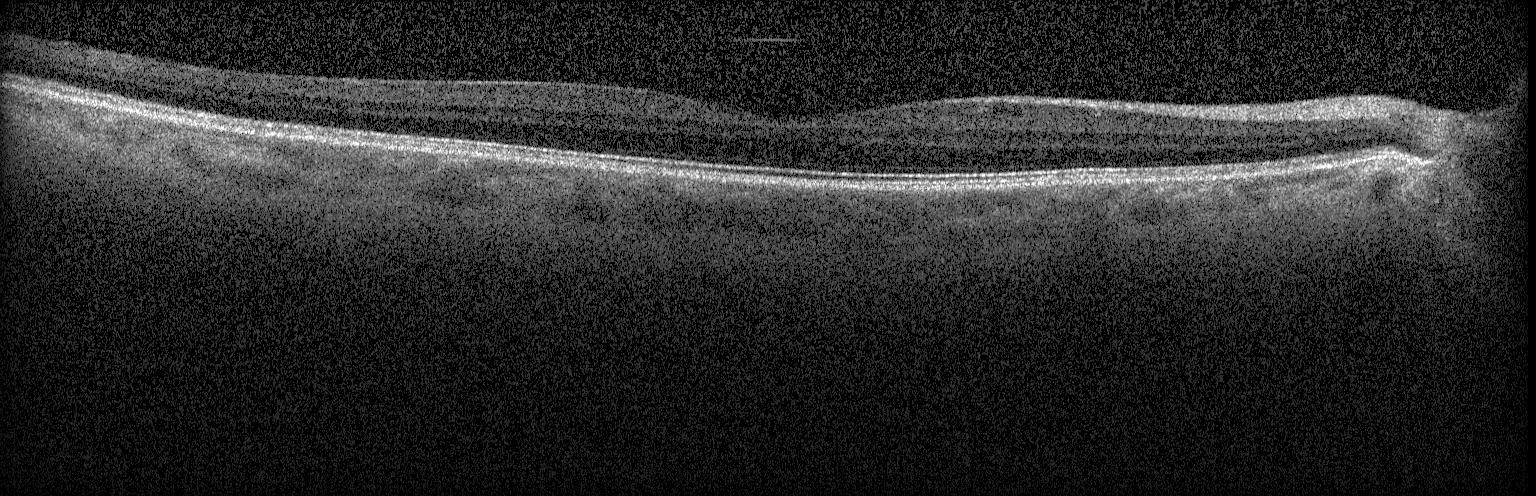
Optical coherence tomography scan. This B-scan demonstrates no CNV, DME, or drusen.